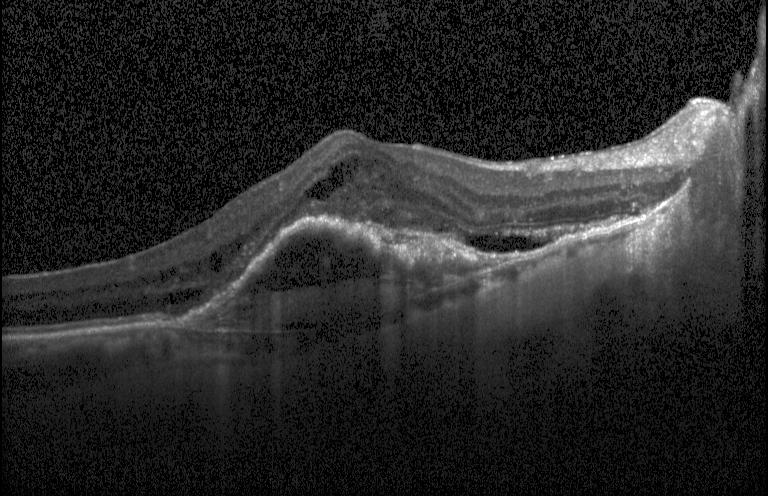
OCT B-scan. Heidelberg Spectralis OCT system. Horizontal scan through the fovea.
The scan shows choroidal neovascularization (CNV).